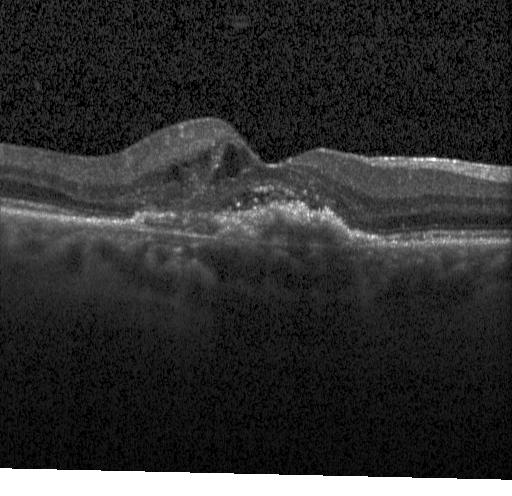

Optical coherence tomography scan, Heidelberg Spectralis OCT system, spectral-domain optical coherence tomography, fovea-centered
A choroidal neovascular membrane.